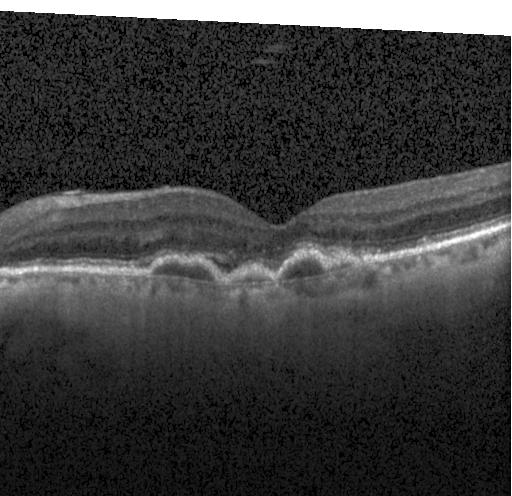
Retinal OCT cross-section showing a choroidal neovascular membrane.